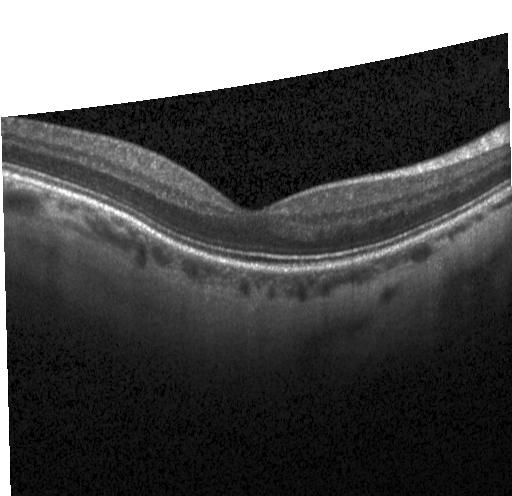
Retinal OCT cross-section. Instrument: Heidelberg Spectralis. Centered on the fovea — Diagnosis: no choroidal neovascularization, no diabetic macular edema, and no drusen.